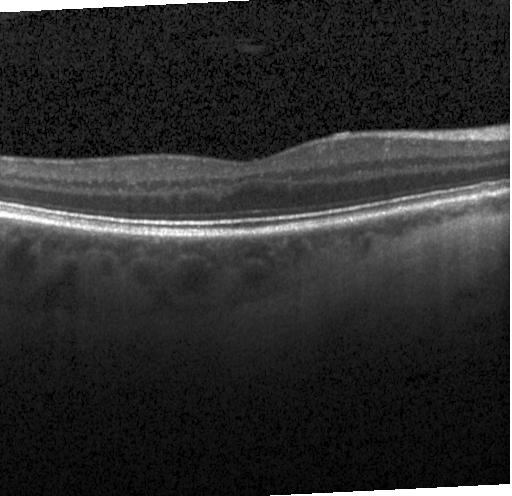 Retinal OCT B-scan. Spectral-domain optical coherence tomography. Assessment: no CNV, no DME, and no drusen.